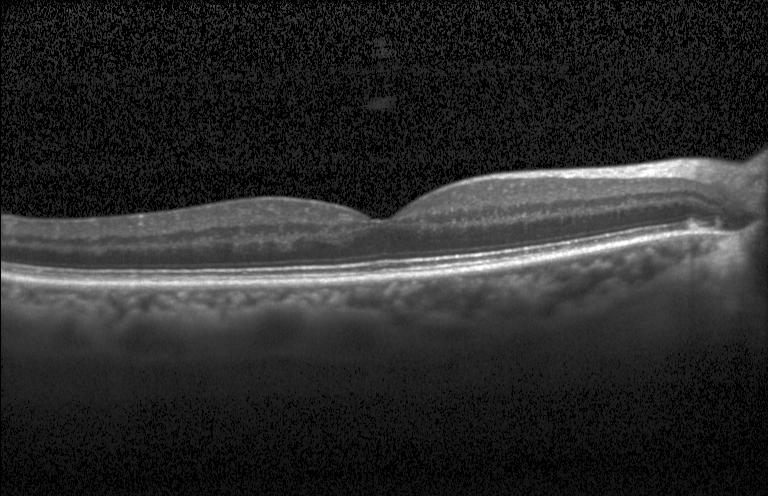

The scan shows no evidence of CNV, DME, or drusen.